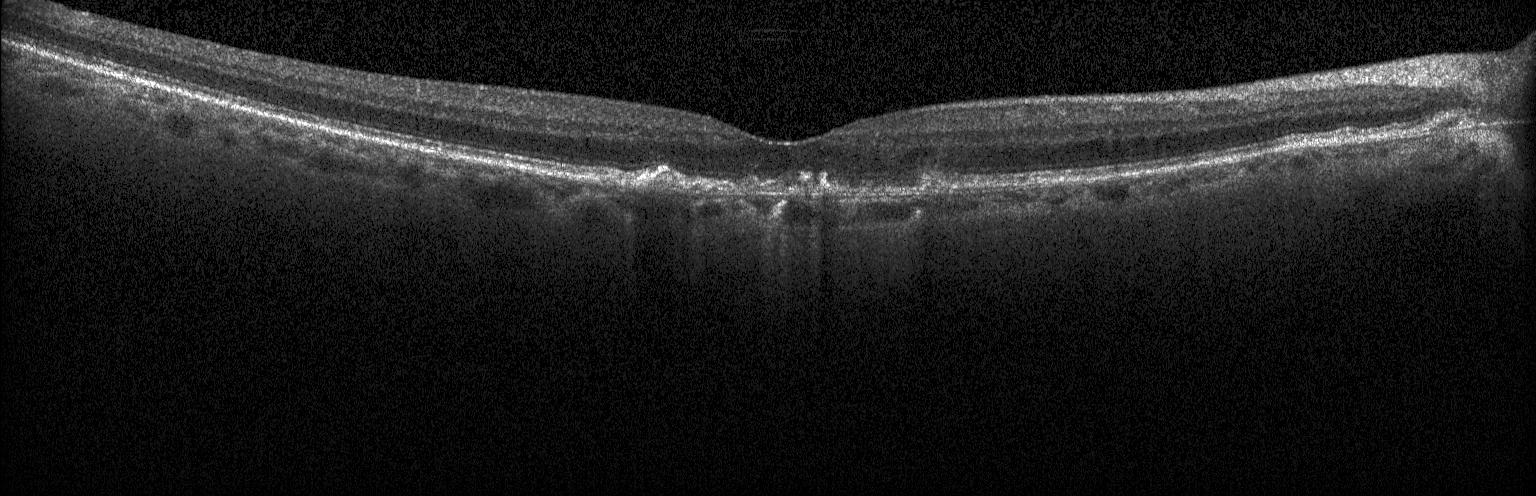 Assessment: sub-RPE drusenoid deposits.